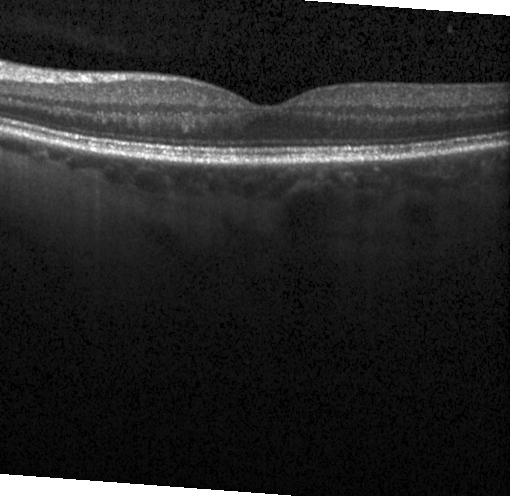

Spectral-domain OCT. Optical coherence tomography scan. Macular scan
Assessment: no CNV, no DME, and no drusen.